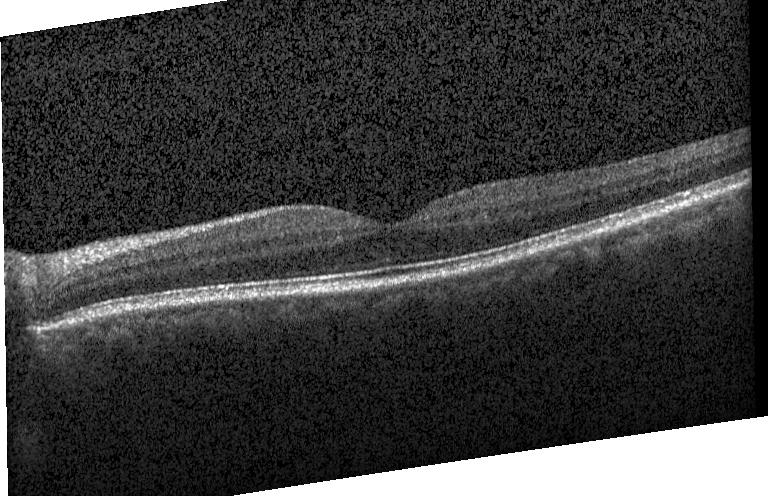
OCT scan showing no choroidal neovascularization, diabetic macular edema, or drusen.